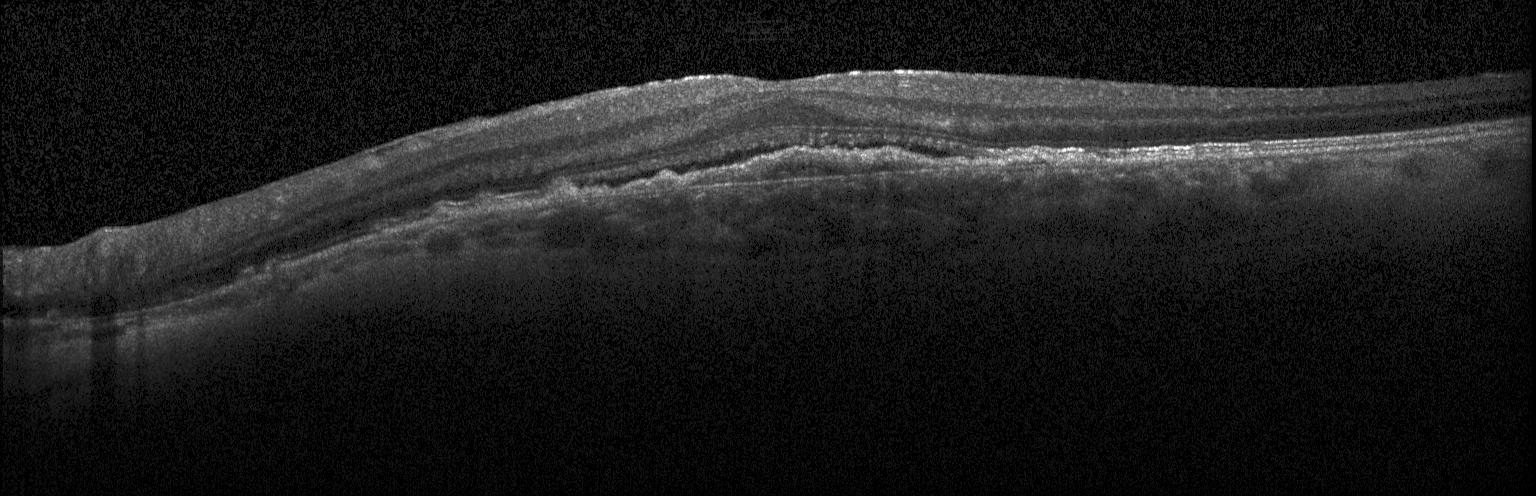

Retinal OCT B-scan.
Finding: choroidal neovascularization.